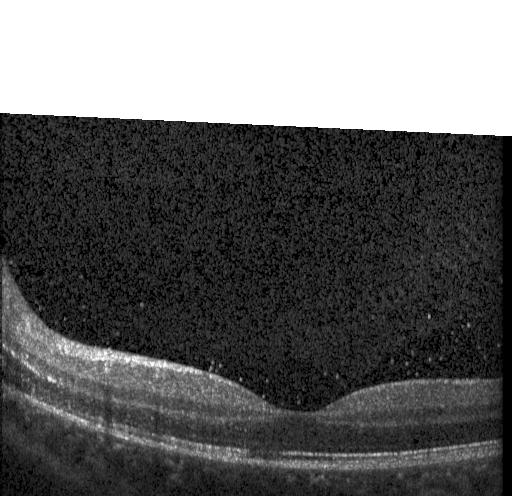
Heidelberg Spectralis · optical coherence tomography B-scan · horizontal scan through the fovea · SD-OCT
Impression: no evidence of choroidal neovascularization, diabetic macular edema, or drusen.